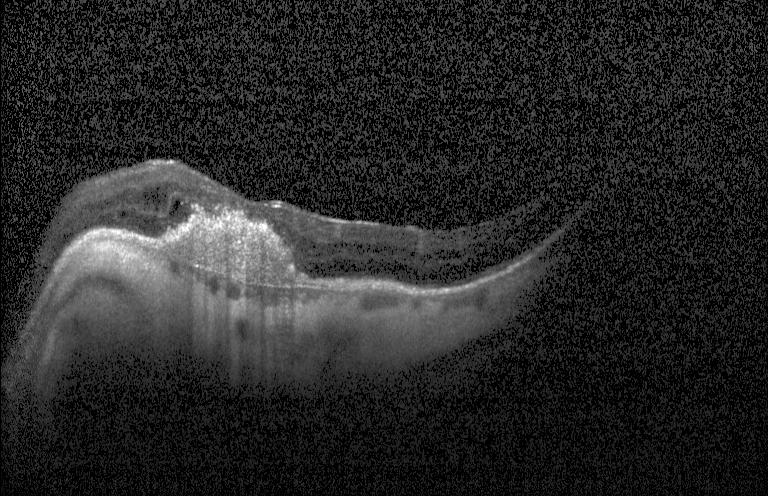 Retinal OCT cross-section · spectral-domain optical coherence tomography — Macular OCT: a choroidal neovascular membrane.